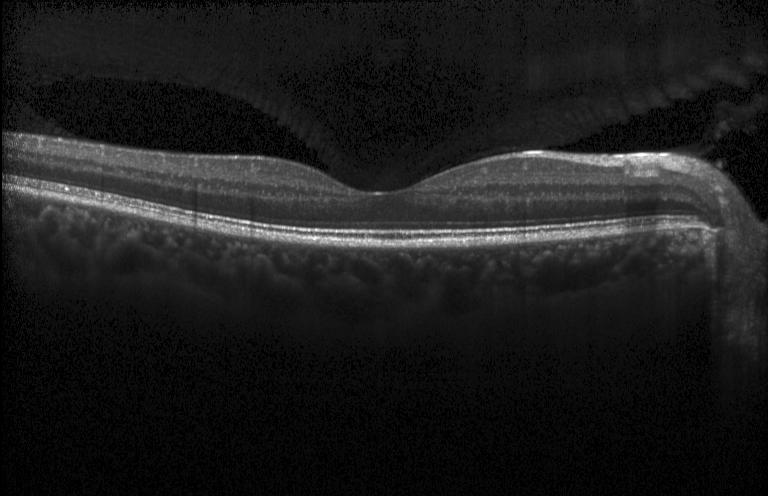 OCT finding: no evidence of choroidal neovascularization, diabetic macular edema, or drusen.